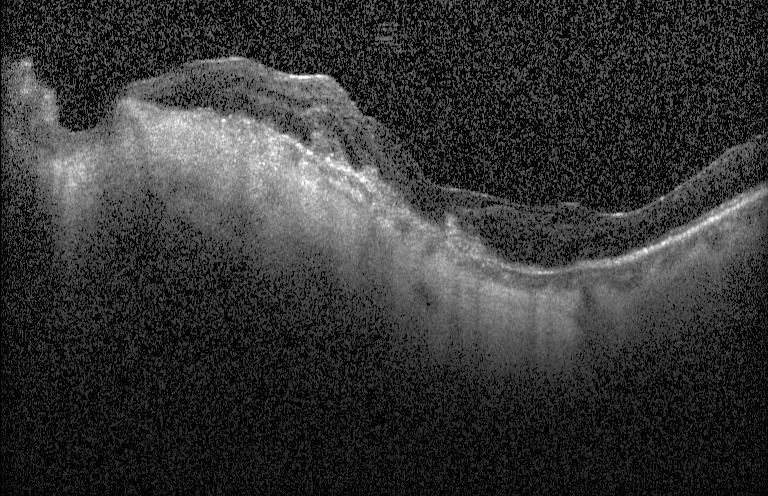

Spectral-domain optical coherence tomography · Heidelberg Spectralis OCT system · retinal OCT cross-section · through the macula. Finding: choroidal neovascularization.